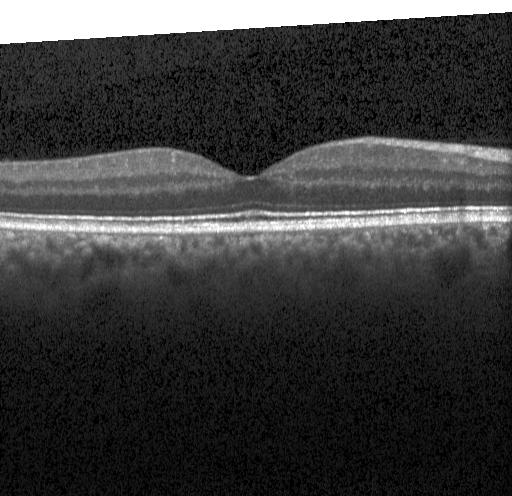 OCT line scan.
The scan shows neither CNV, DME, nor drusen.